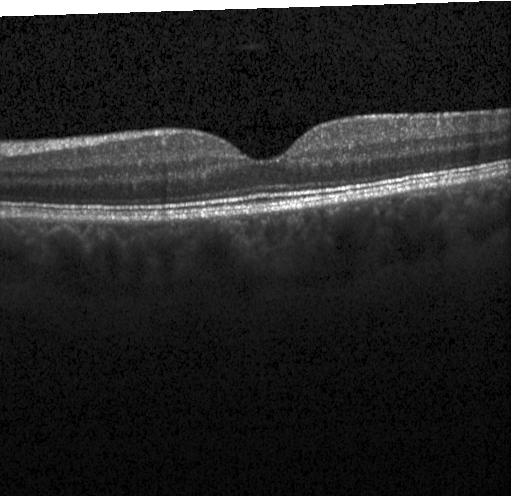
Retinal OCT B-scan, spectral-domain optical coherence tomography, macular scan. OCT finding: no choroidal neovascularization, diabetic macular edema, or drusen.